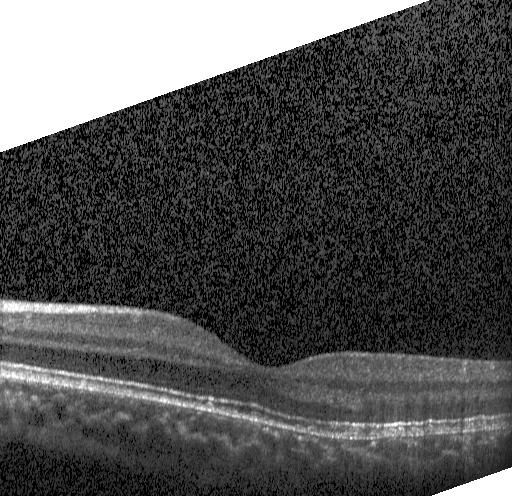 Finding: no choroidal neovascularization, no diabetic macular edema, and no drusen.